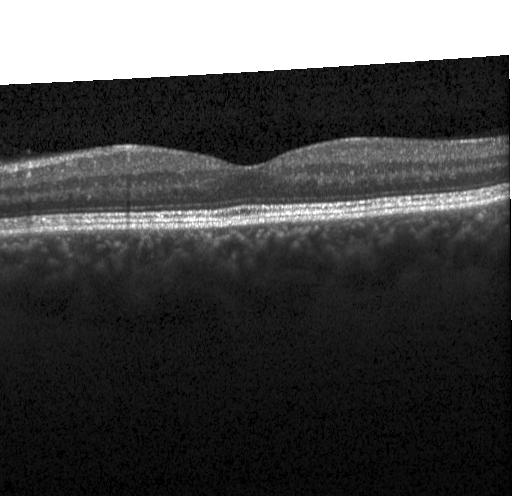 Optical coherence tomography B-scan.
No evidence of choroidal neovascularization, diabetic macular edema, or drusen.